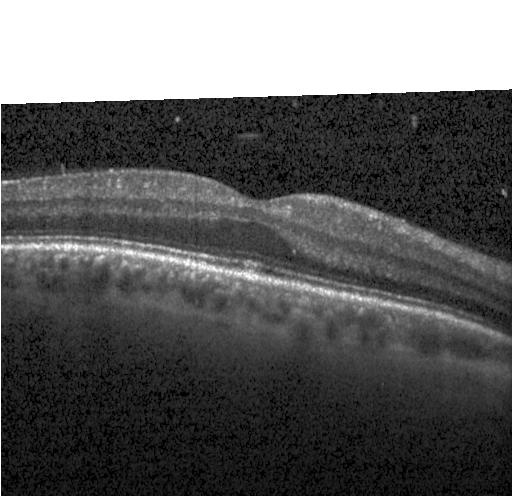
Assessment: no choroidal neovascularization, diabetic macular edema, or drusen.